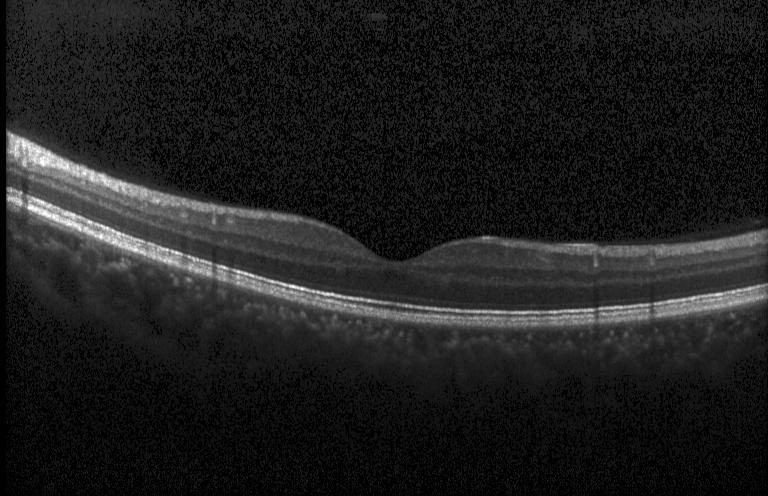 Diagnosis: no evidence of choroidal neovascularization, diabetic macular edema, or drusen.